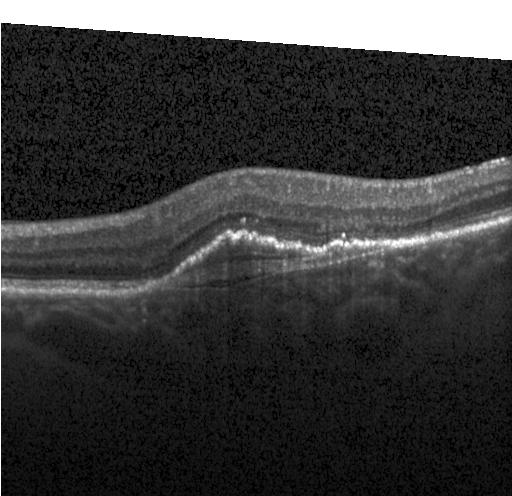

Retinal OCT cross-section · Heidelberg Spectralis · spectral-domain optical coherence tomography.
Impression: a choroidal neovascular membrane.